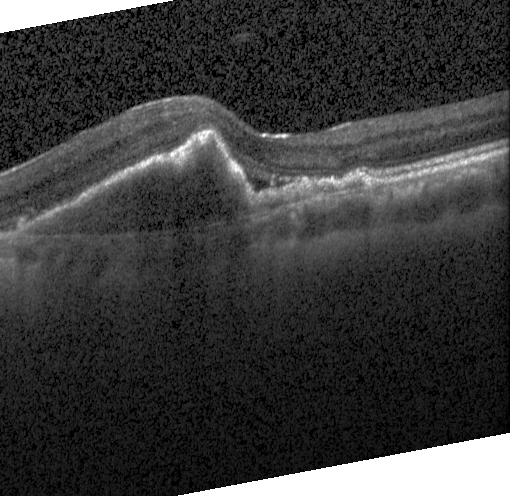 Retinal OCT cross-section; spectral-domain OCT; macular scan; Heidelberg Spectralis
Diagnosis: CNV.